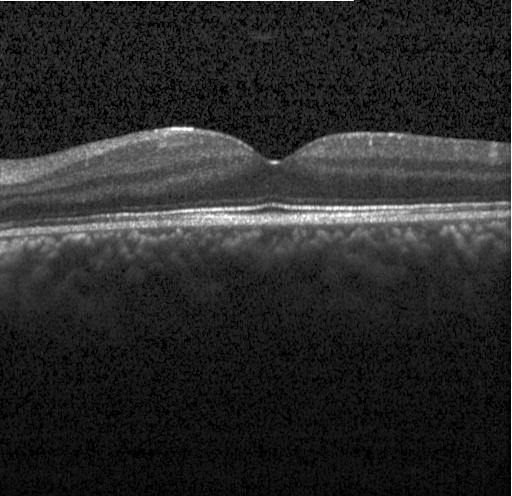
Optical coherence tomography B-scan; SD-OCT; fovea-centered.
Impression: no choroidal neovascularization, no diabetic macular edema, and no drusen.